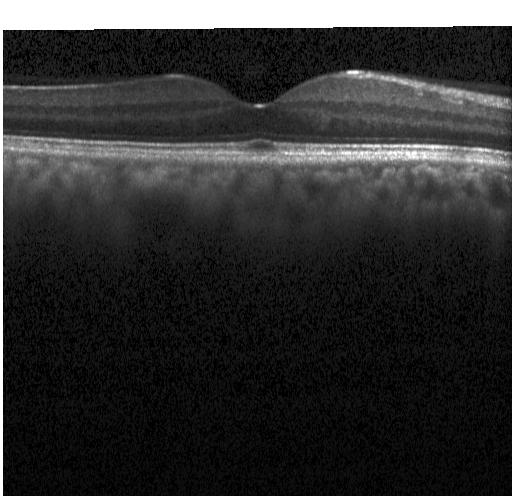 Diagnosis: no CNV, DME, or drusen.